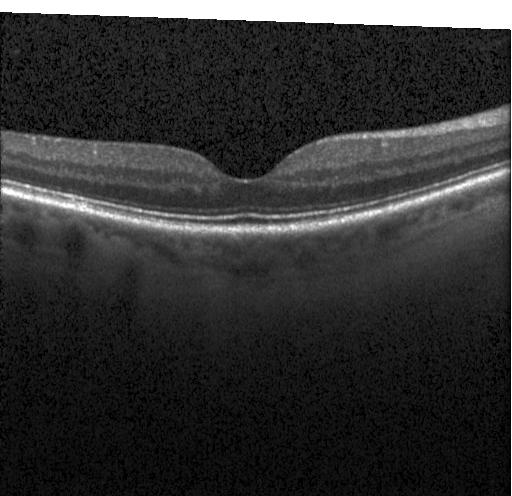 Impression: no evidence of choroidal neovascularization, diabetic macular edema, or drusen.